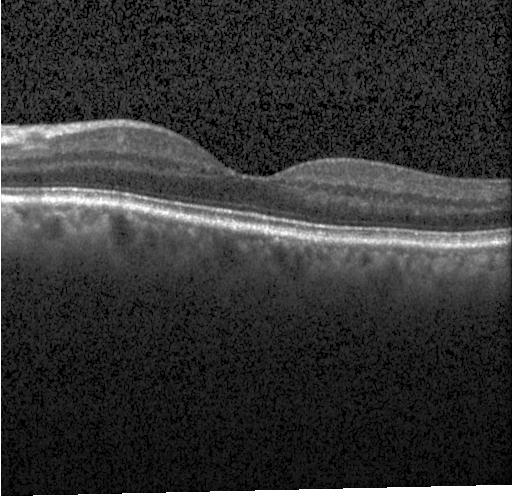 Spectral-domain OCT · OCT line scan
Dx: no choroidal neovascularization, no diabetic macular edema, and no drusen.